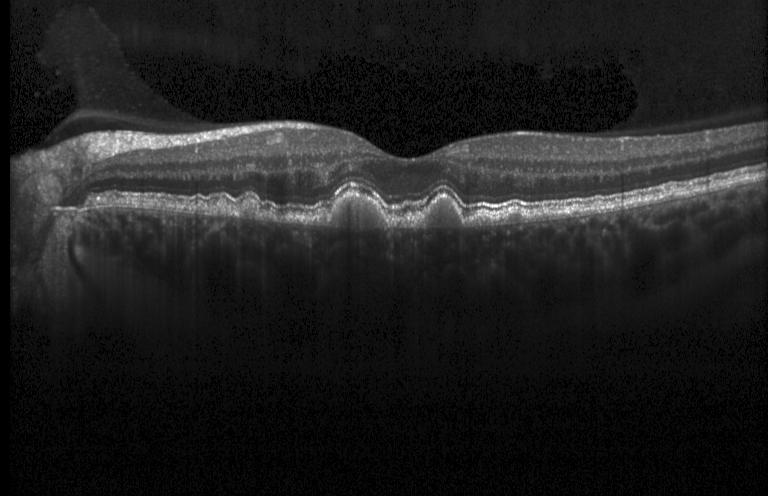
Finding: multiple drusen.